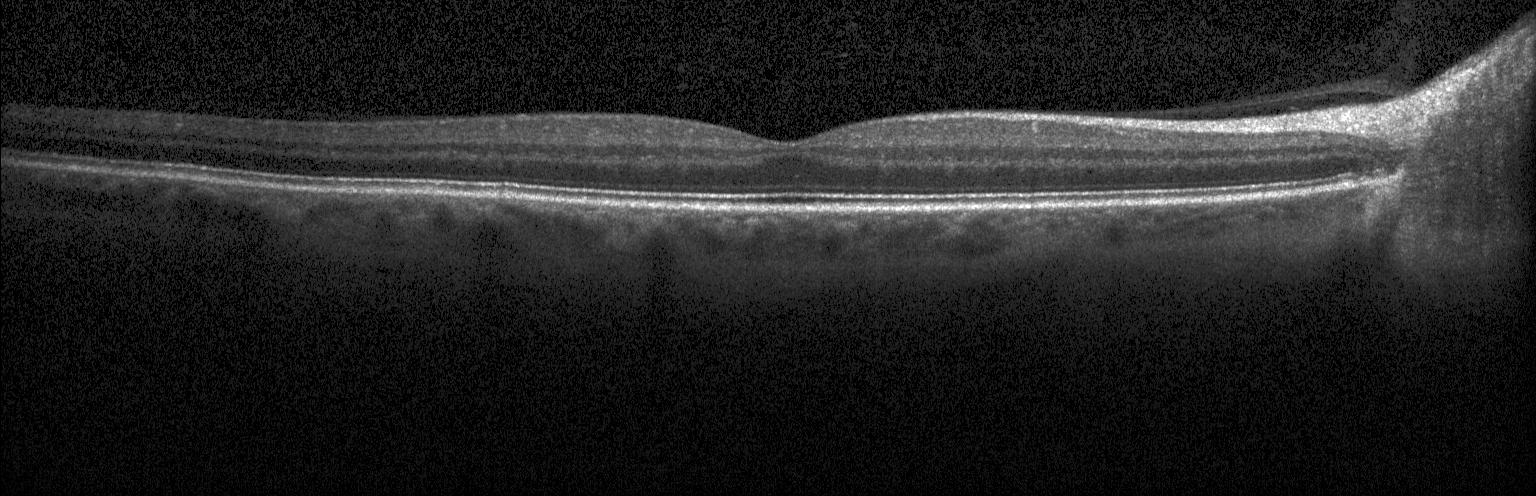 Retinal OCT cross-section.
No evidence of CNV, DME, or drusen.